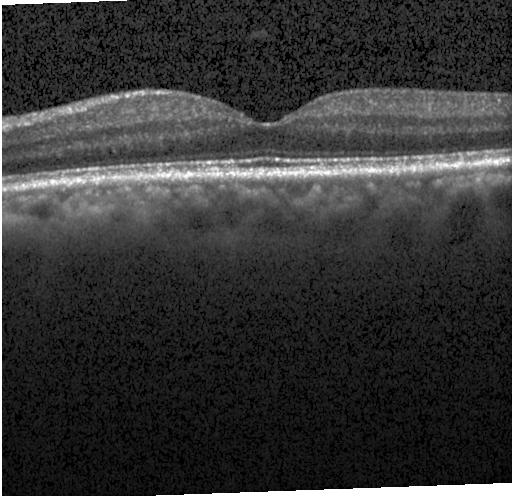

OCT B-scan. This B-scan demonstrates no choroidal neovascularization, diabetic macular edema, or drusen.